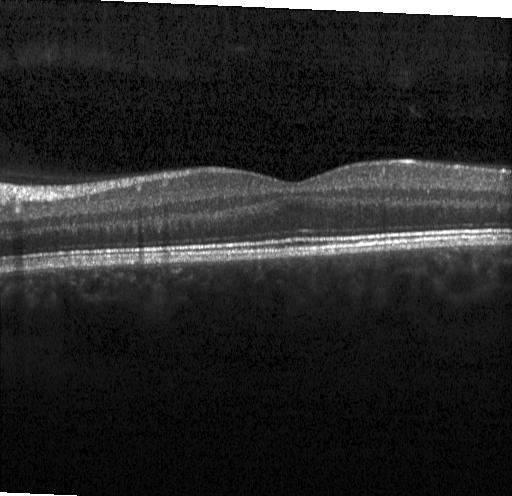
Optical coherence tomography scan.
This B-scan demonstrates neither choroidal neovascularization, diabetic macular edema, nor drusen.